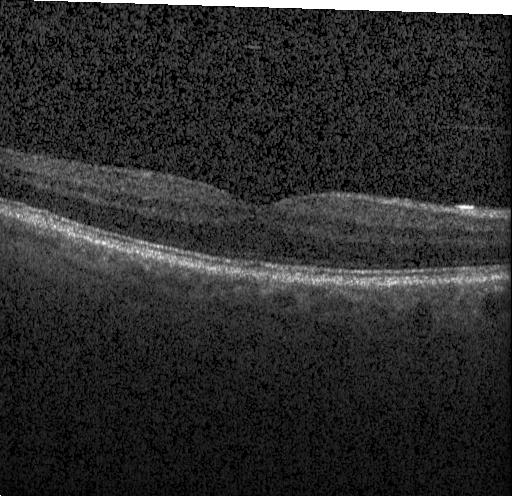 Assessment: no CNV, DME, or drusen.